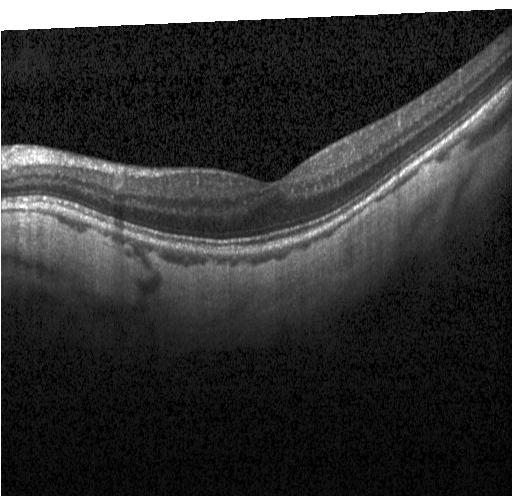
No evidence of CNV, DME, or drusen.